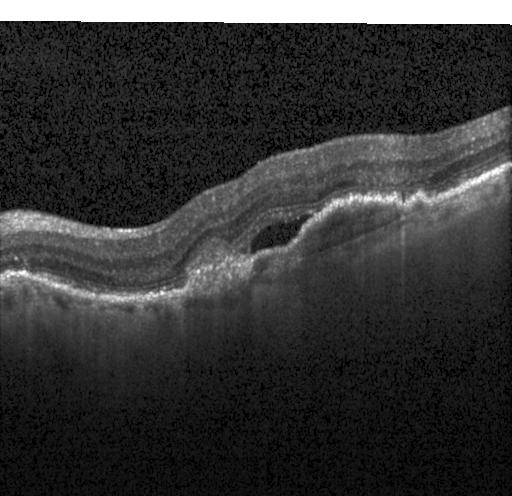 Macular scan. OCT line scan. Heidelberg Spectralis. Spectral-domain OCT. Finding: a choroidal neovascular membrane.